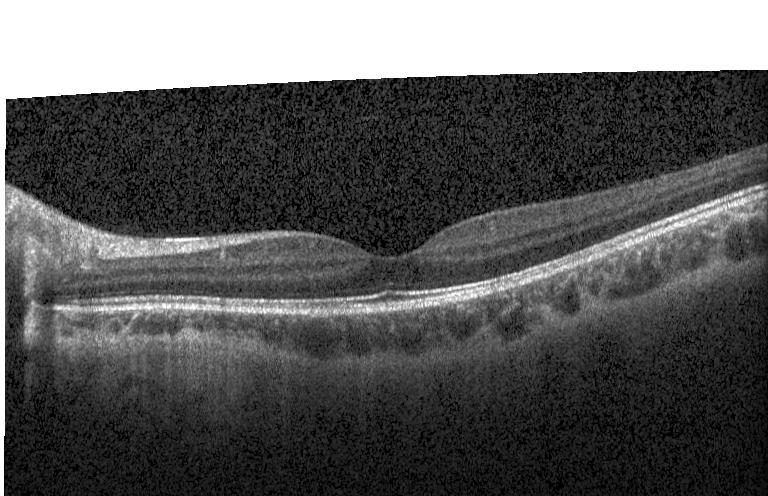

Horizontal scan through the fovea · spectral-domain OCT · acquired on a Heidelberg Spectralis · OCT B-scan — Diagnosis: no evidence of CNV, DME, or drusen.